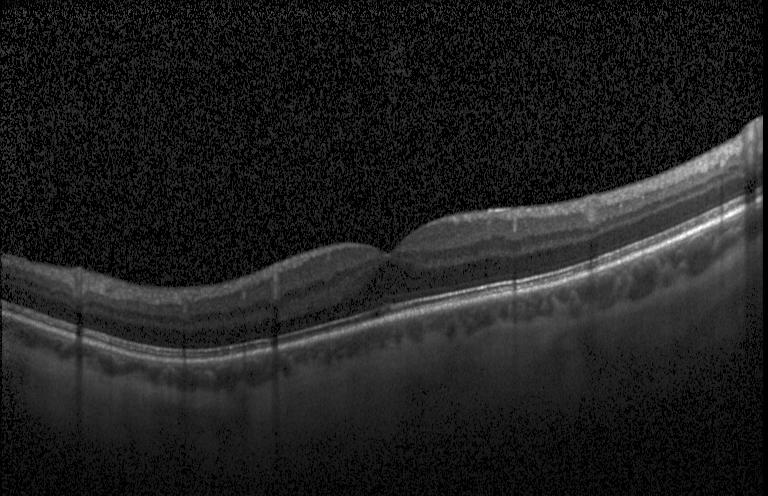

Centered on the fovea, retinal OCT B-scan
This B-scan demonstrates no choroidal neovascularization, diabetic macular edema, or drusen.